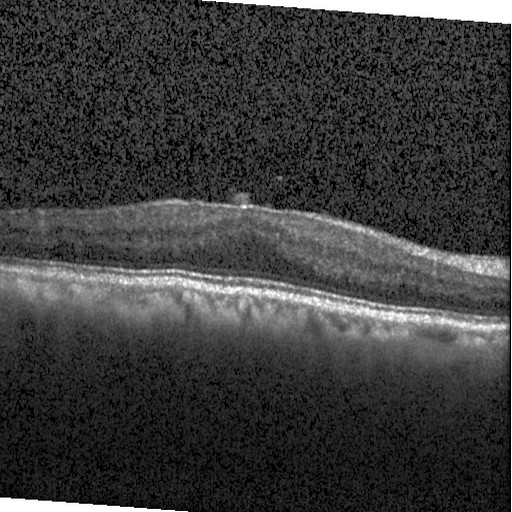 Retinal OCT cross-section. Diagnosis: diabetic macular edema (DME).